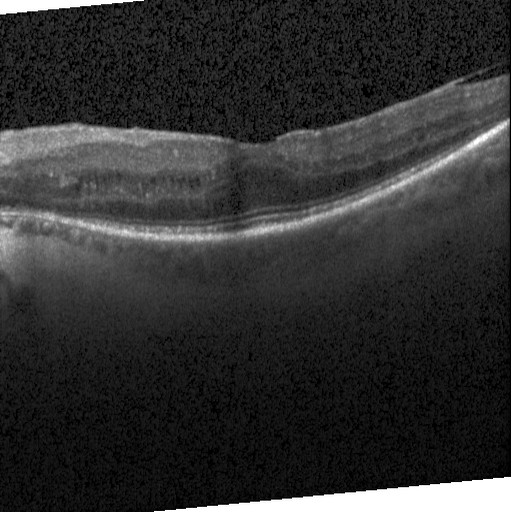 SD-OCT · instrument: Heidelberg Spectralis · optical coherence tomography B-scan — Macular OCT: diabetic macular edema.